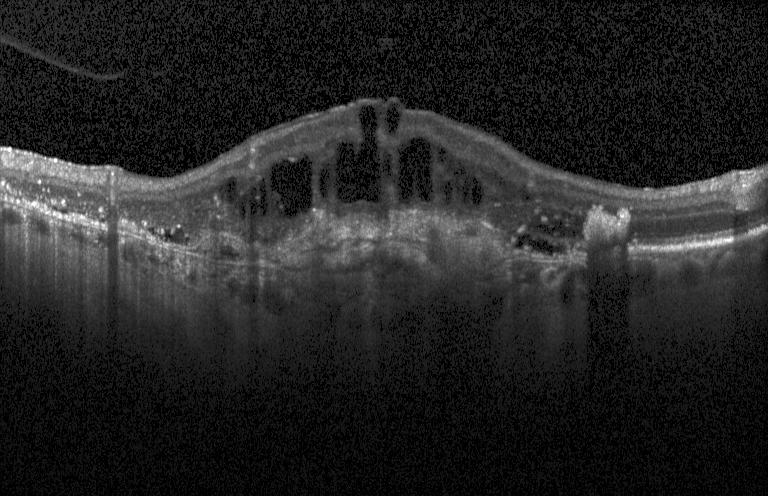 OCT scan showing choroidal neovascularization (CNV).